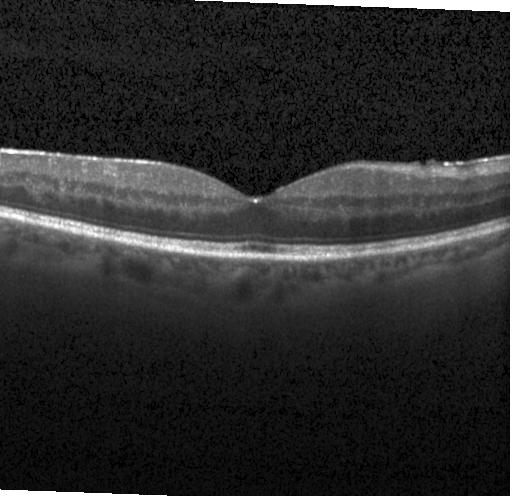 OCT line scan; centered on the fovea — Assessment: neither choroidal neovascularization, diabetic macular edema, nor drusen.